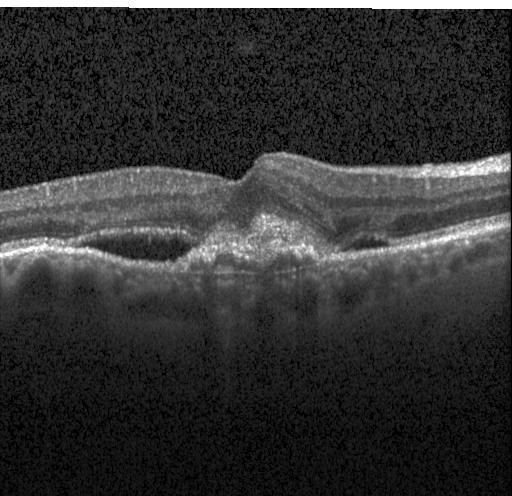
Optical coherence tomography scan. Diagnosis: a choroidal neovascular membrane.